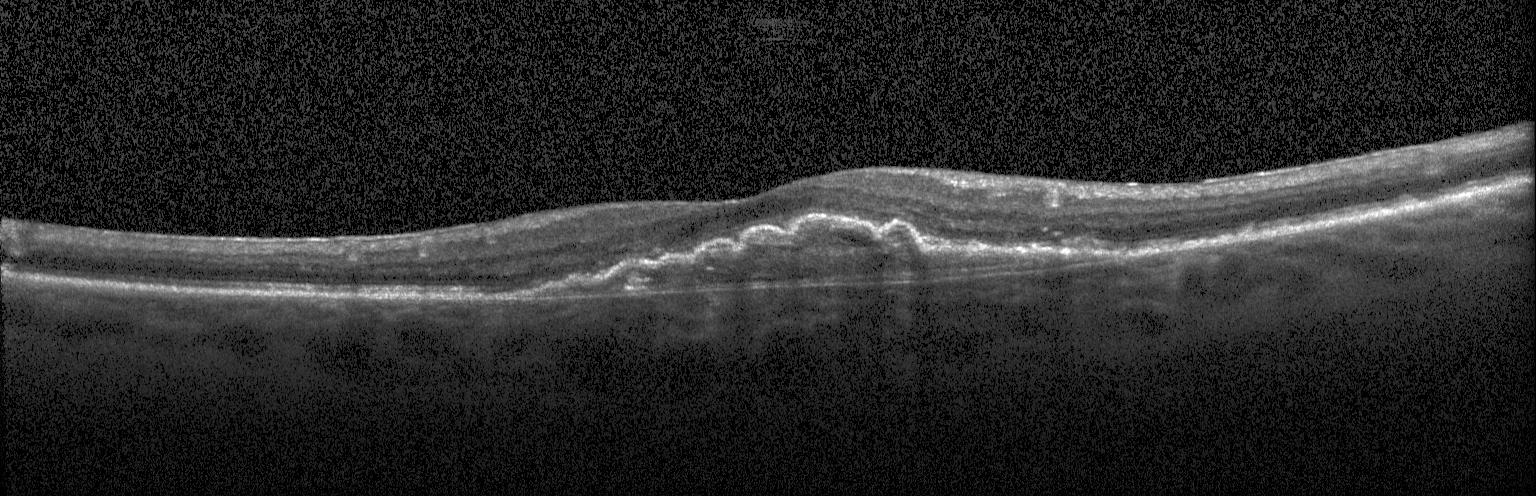

Impression: a choroidal neovascular membrane.